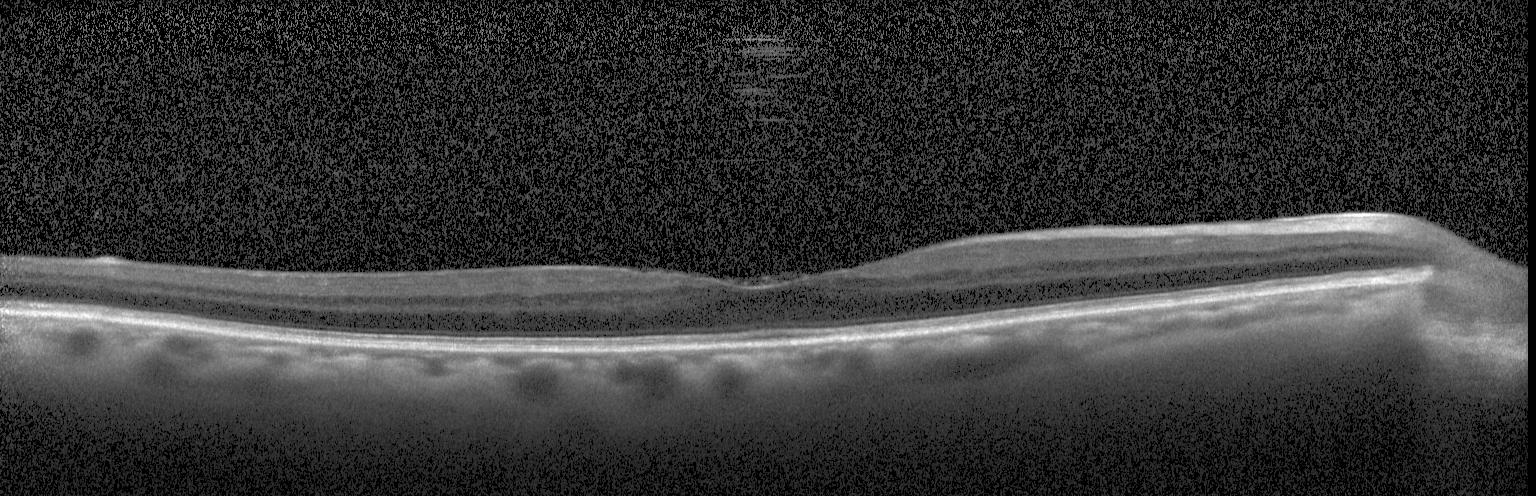

Heidelberg Spectralis · centered on the fovea · retinal OCT B-scan · spectral-domain optical coherence tomography. This B-scan demonstrates neither choroidal neovascularization, diabetic macular edema, nor drusen.